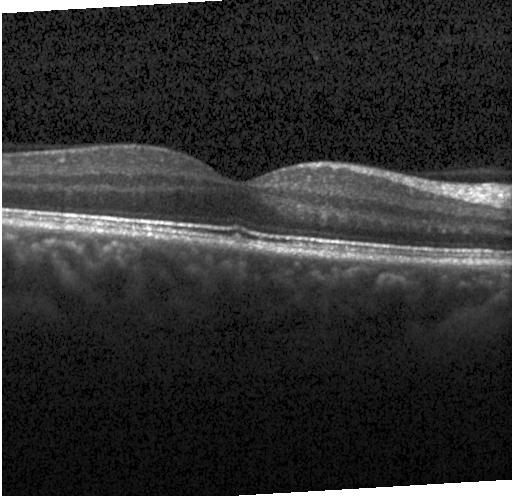 Optical coherence tomography scan — Impression: multiple drusen.